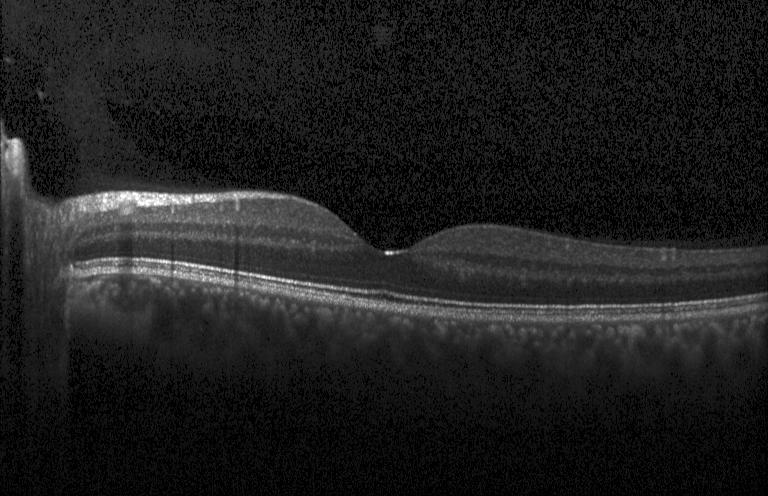
Heidelberg Spectralis OCT system · spectral-domain OCT · retinal OCT B-scan · through the macula. Finding: no CNV, no DME, and no drusen.